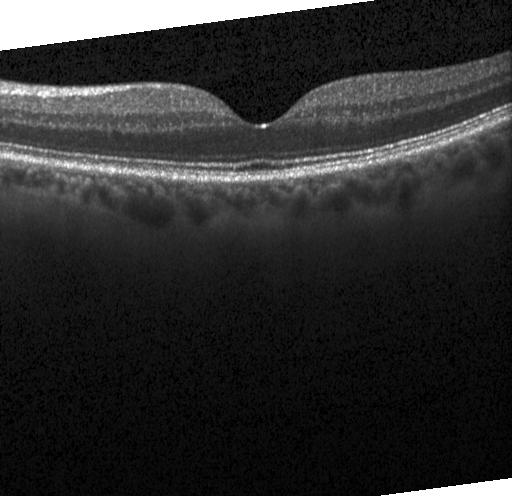

Macular scan. Spectral-domain OCT. Retinal OCT cross-section. Acquired on a Heidelberg Spectralis
Finding: no evidence of choroidal neovascularization, diabetic macular edema, or drusen.